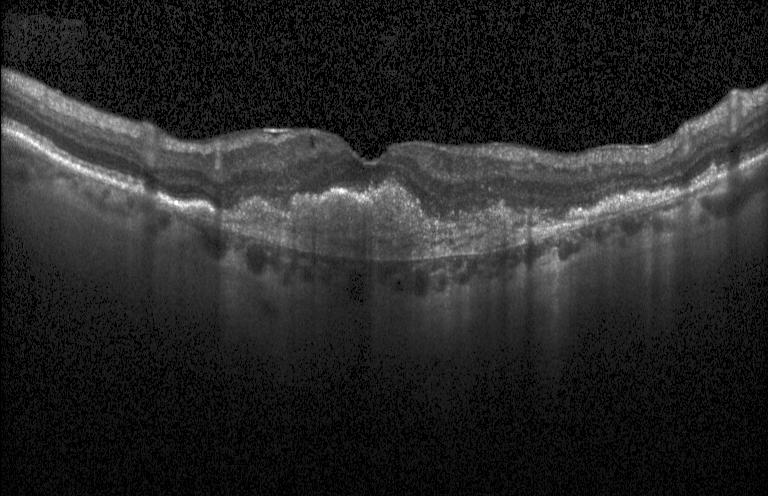
Acquired on a Heidelberg Spectralis; OCT line scan; SD-OCT; through the macula
Impression: a choroidal neovascular membrane.